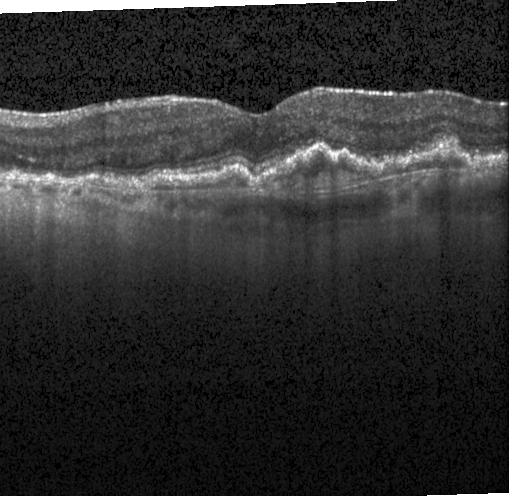 Macular OCT: CNV.